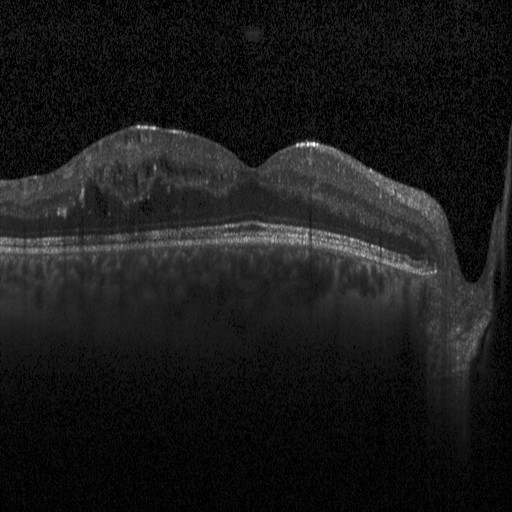 Diagnosis: DME.